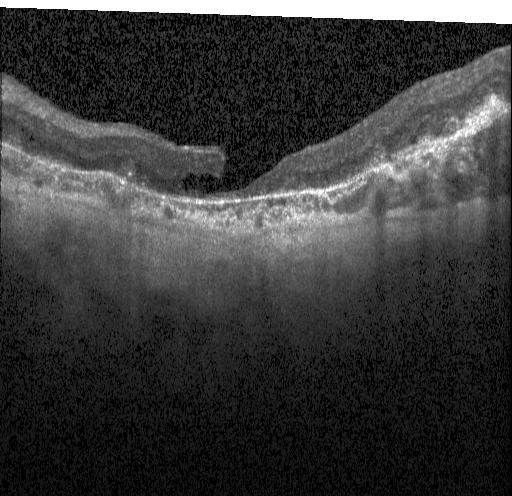 Impression: CNV.